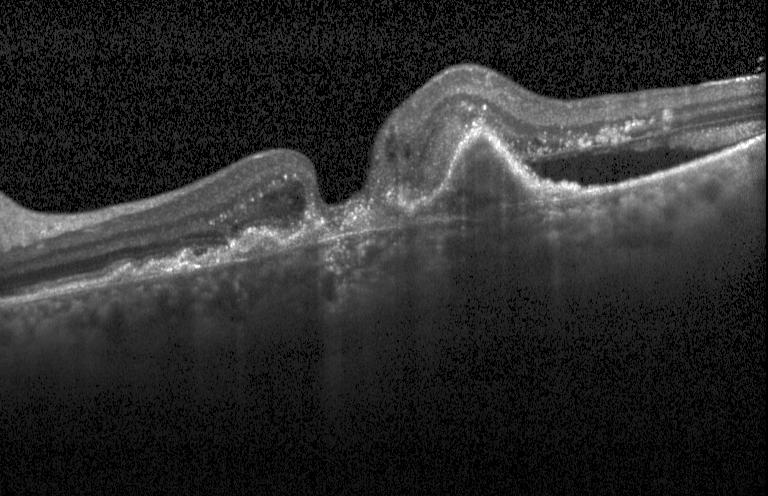
Retinal OCT cross-section.
Impression: CNV.